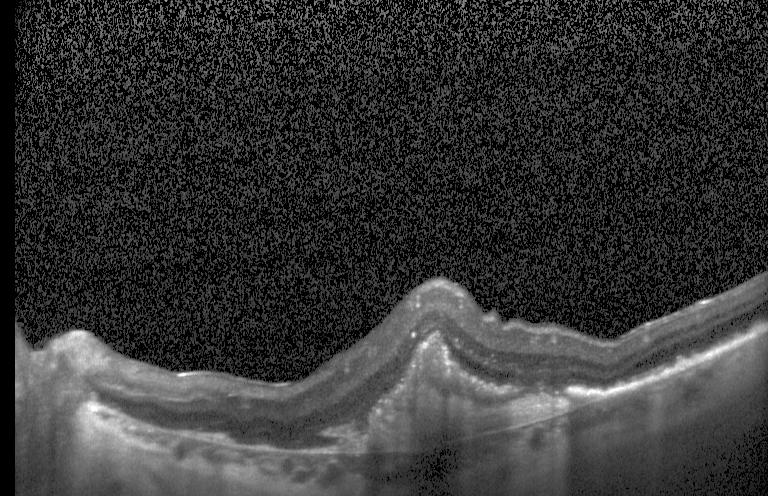
SD-OCT · retinal OCT B-scan. The scan shows choroidal neovascularization (CNV).